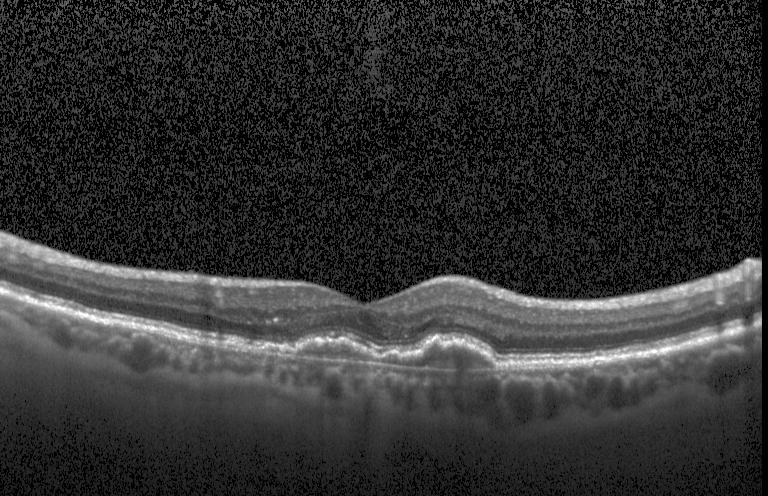
OCT B-scan. Heidelberg Spectralis. Spectral-domain optical coherence tomography. Fovea-centered
The scan shows a choroidal neovascular membrane.